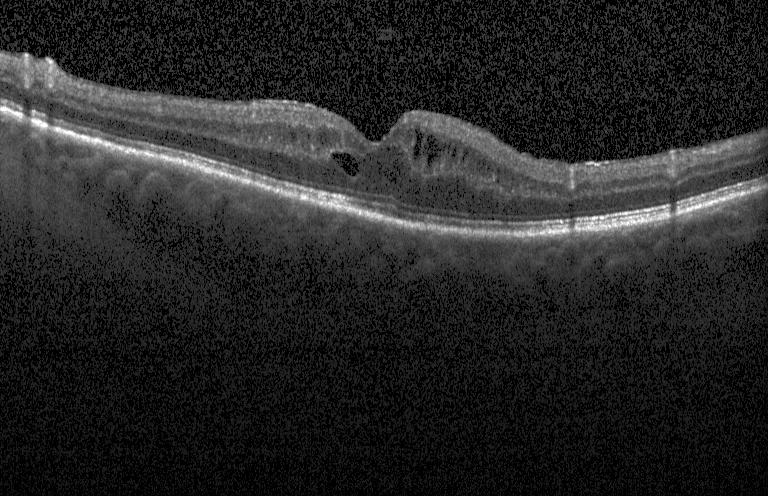
Spectral-domain OCT, instrument: Heidelberg Spectralis, OCT line scan. The scan shows DME.